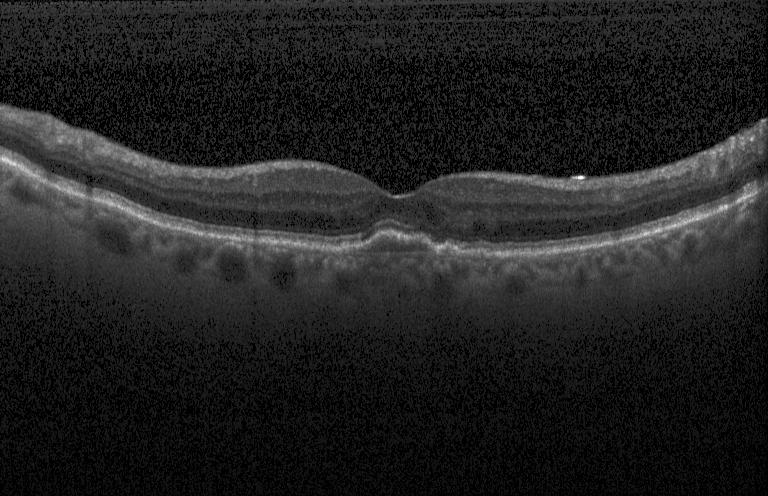
Retinal OCT cross-section — Diagnosis: choroidal neovascularization.